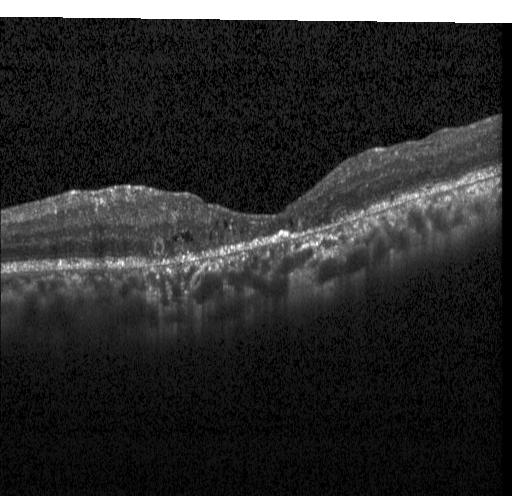 Acquired on a Heidelberg Spectralis. Through the macula. Spectral-domain optical coherence tomography. Retinal OCT B-scan. Assessment: a choroidal neovascular membrane.